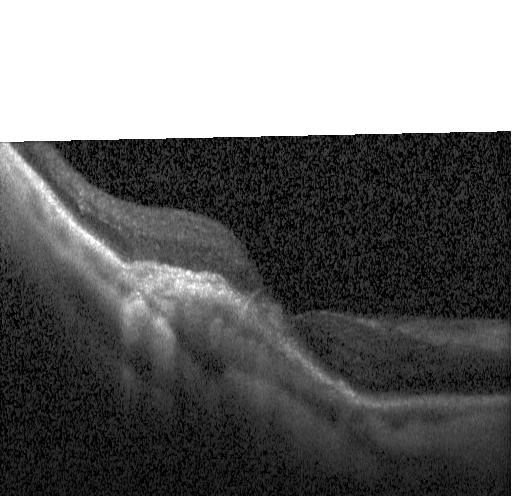
Spectral-domain OCT, Heidelberg Spectralis, retinal OCT B-scan
This B-scan demonstrates choroidal neovascularization.